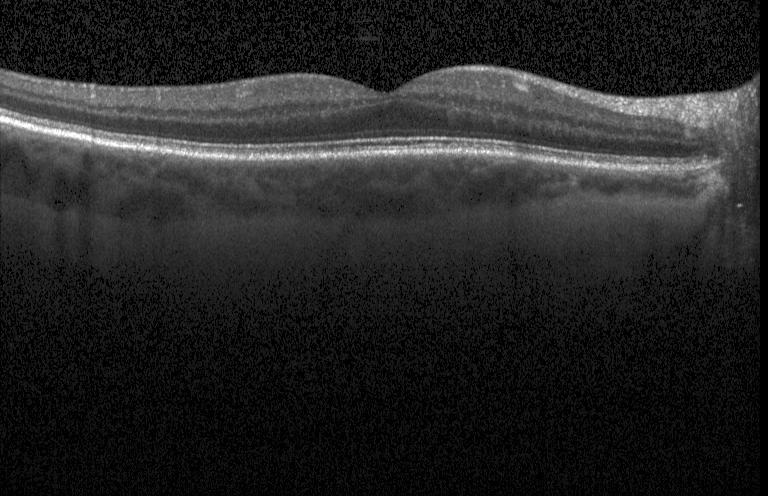

Macular OCT: no choroidal neovascularization, no diabetic macular edema, and no drusen.